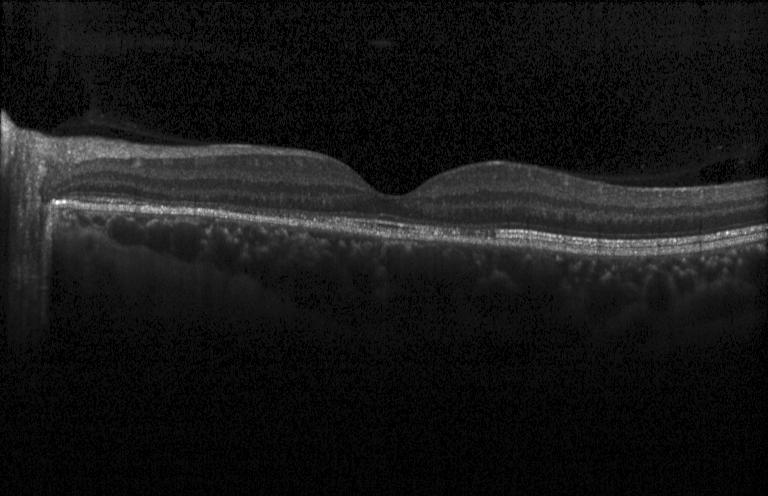
Macular scan · Heidelberg Spectralis · spectral-domain optical coherence tomography · OCT B-scan — Assessment: no CNV, no DME, and no drusen.